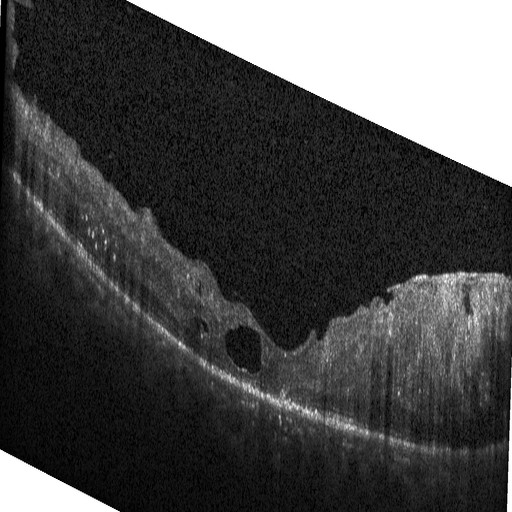
OCT finding: diabetic macular edema.